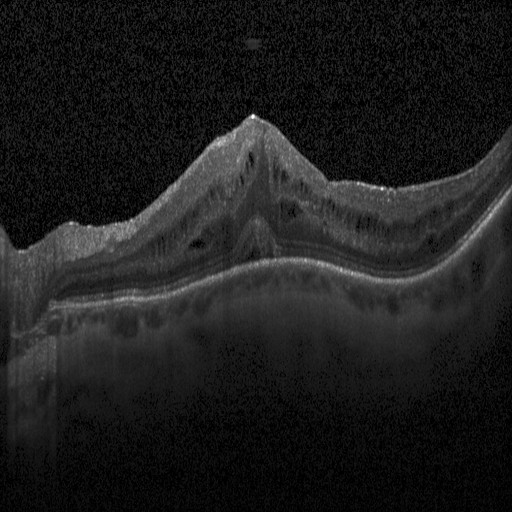

OCT B-scan. Diabetic macular edema.